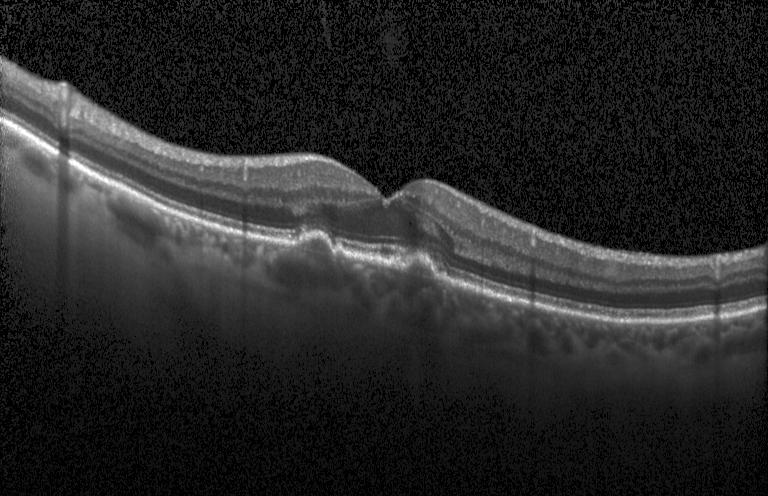
Finding: choroidal neovascularization (CNV).